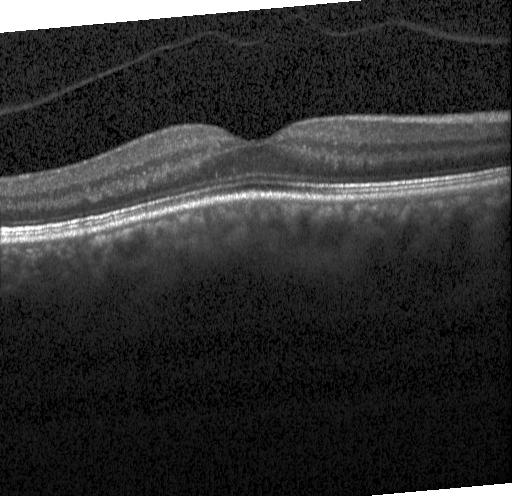 Optical coherence tomography B-scan · spectral-domain optical coherence tomography.
Impression: neither CNV, DME, nor drusen.